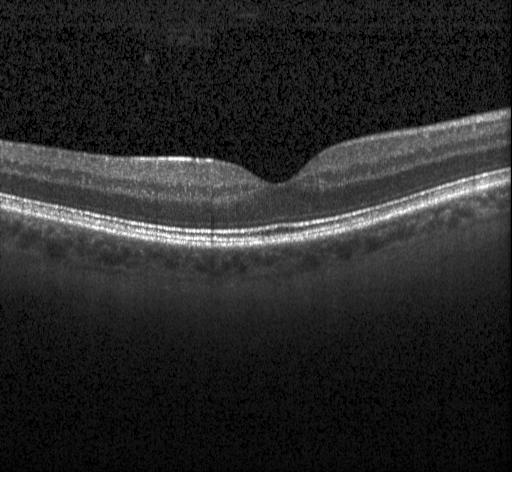
Finding: no evidence of choroidal neovascularization, diabetic macular edema, or drusen.